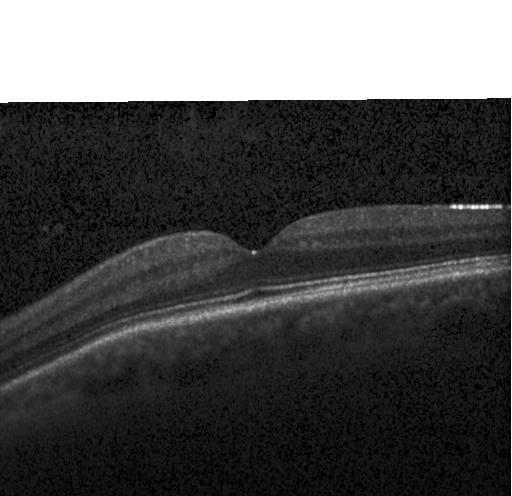

OCT B-scan, Heidelberg Spectralis, centered on the fovea, spectral-domain OCT.
This B-scan demonstrates no choroidal neovascularization, diabetic macular edema, or drusen.